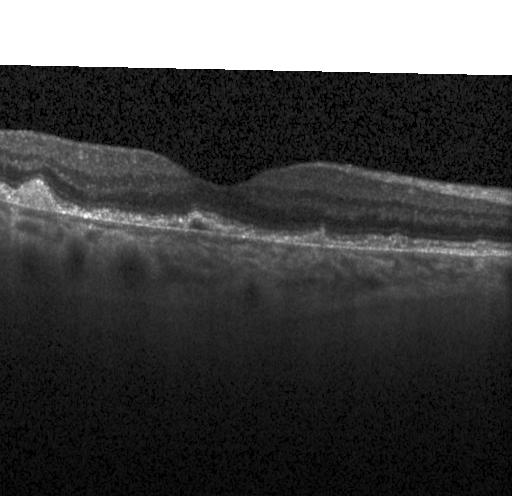

The scan shows choroidal neovascularization.